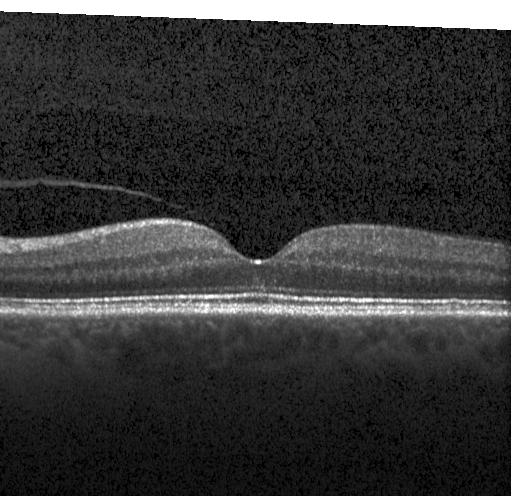

Dx: neither choroidal neovascularization, diabetic macular edema, nor drusen.